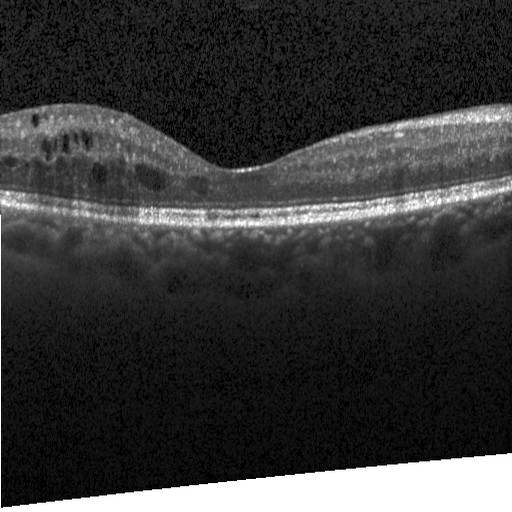

Optical coherence tomography scan. Heidelberg Spectralis OCT system. Fovea-centered. The scan shows diabetic macular edema.